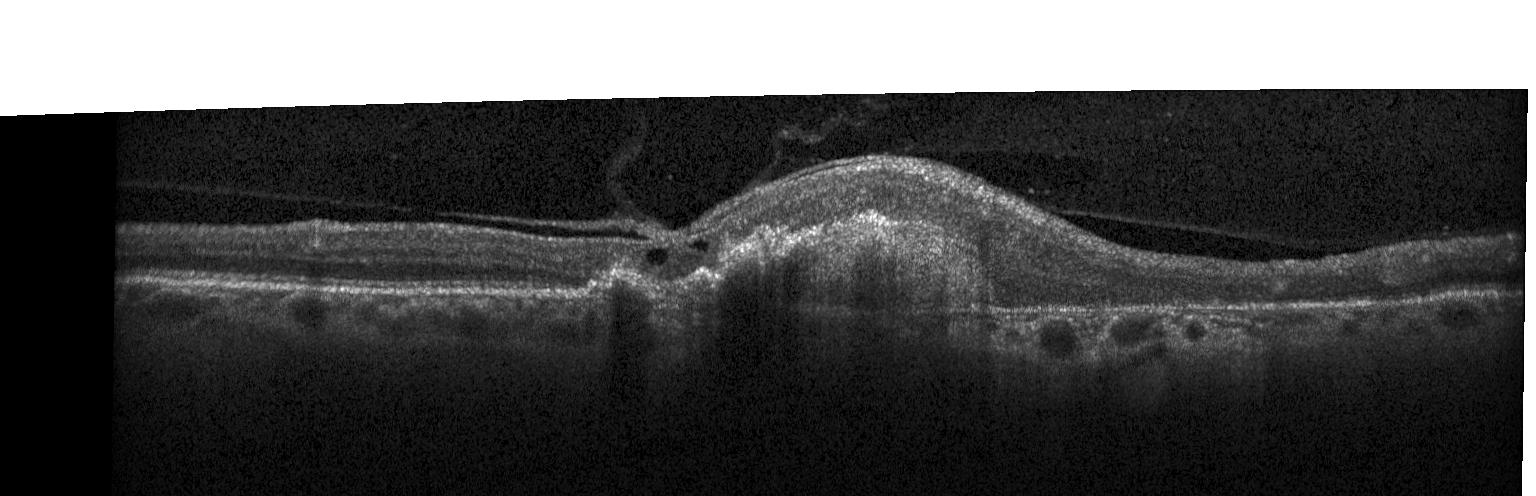 SD-OCT; optical coherence tomography scan; instrument: Heidelberg Spectralis.
Diagnosis: a choroidal neovascular membrane.